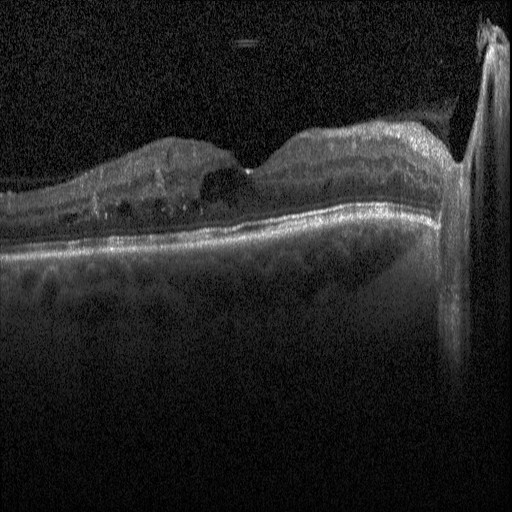 Acquired on a Heidelberg Spectralis, retinal OCT B-scan, horizontal scan through the fovea
OCT finding: diabetic macular edema.